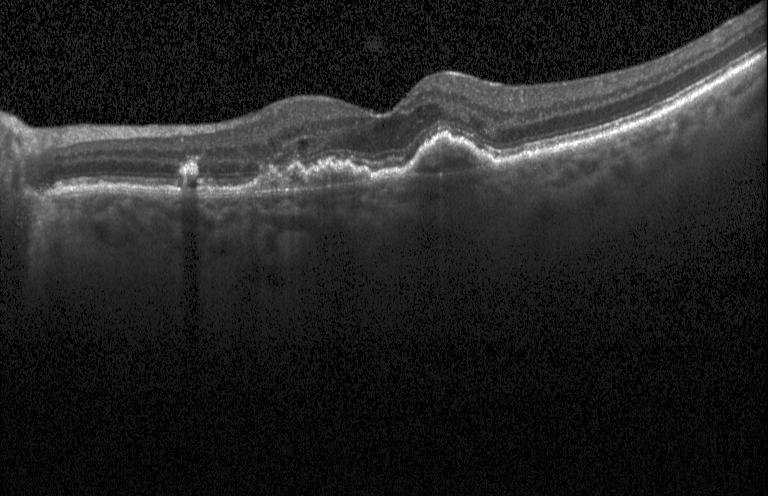 SD-OCT. Retinal OCT B-scan. Macular OCT: a choroidal neovascular membrane.